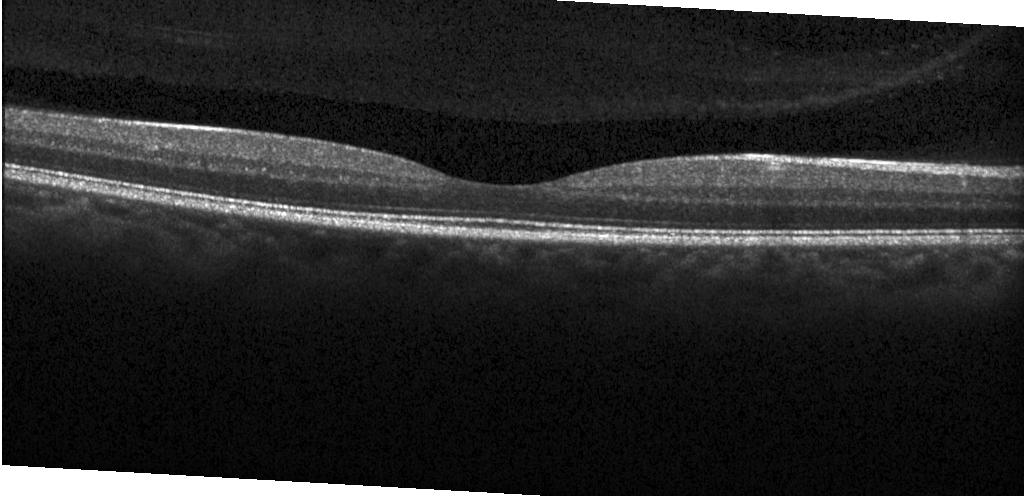
Fovea-centered; optical coherence tomography B-scan
Macular OCT: no CNV, no DME, and no drusen.